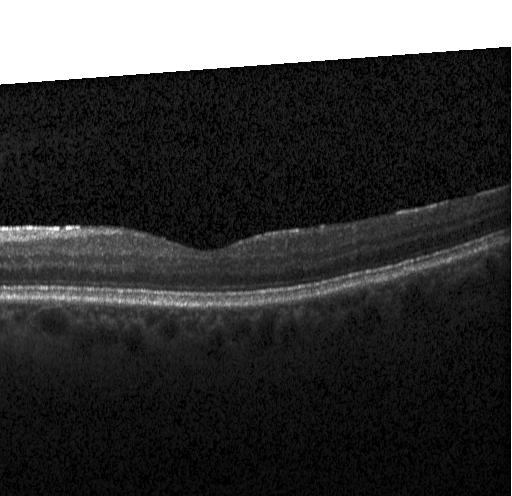
Through the macula, OCT B-scan
Assessment: neither choroidal neovascularization, diabetic macular edema, nor drusen.